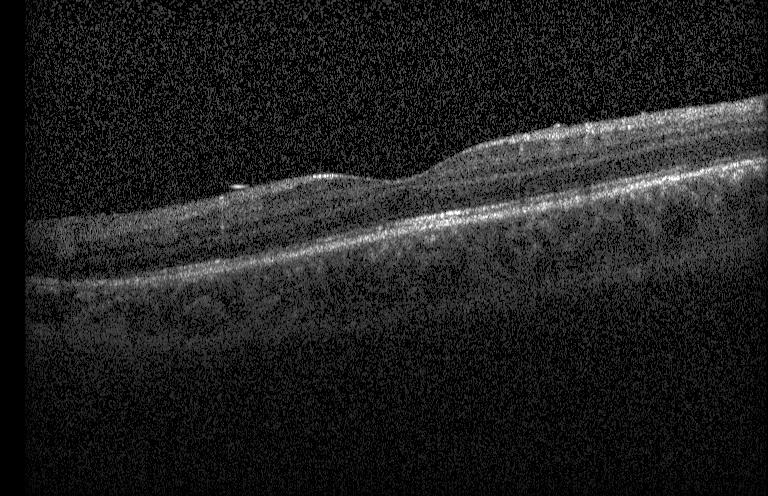
Centered on the fovea, OCT line scan
Dx: no choroidal neovascularization, no diabetic macular edema, and no drusen.